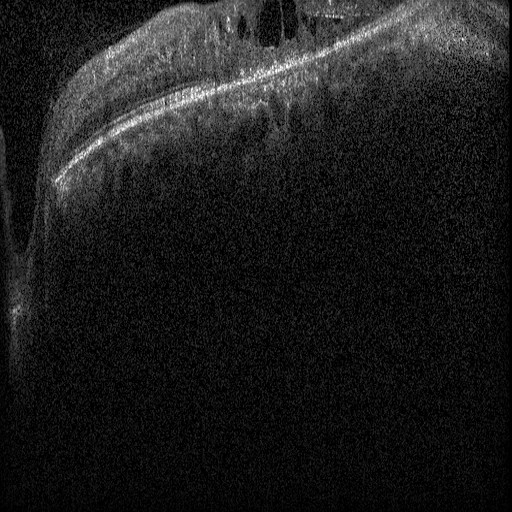
Spectral-domain OCT; through the macula; instrument: Heidelberg Spectralis; optical coherence tomography scan
This B-scan demonstrates DME.